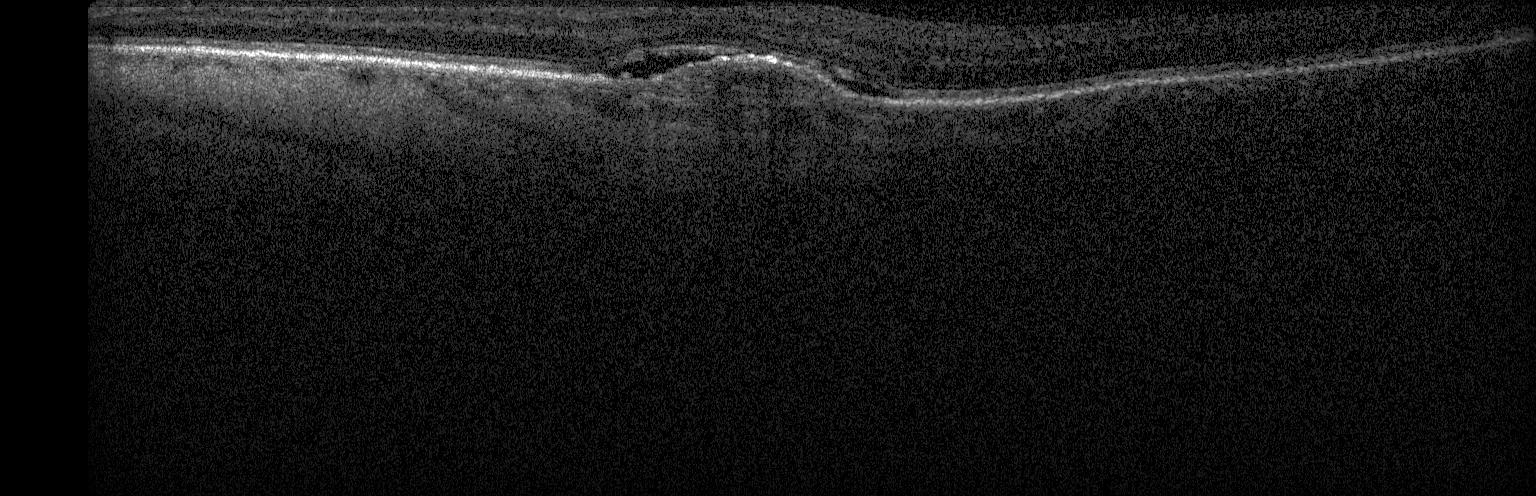 Finding: a choroidal neovascular membrane.